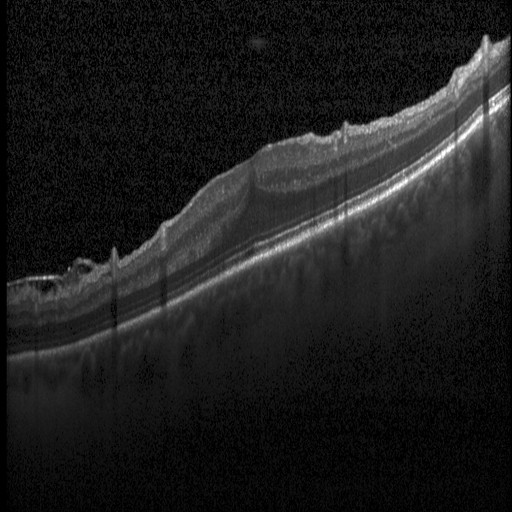
Optical coherence tomography B-scan · macular scan · instrument: Heidelberg Spectralis.
DME.